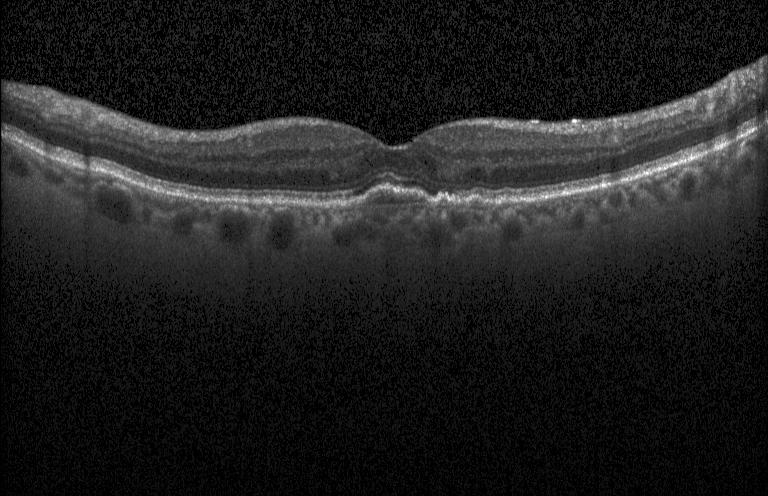 Retinal OCT cross-section; centered on the fovea; spectral-domain OCT.
Assessment: a choroidal neovascular membrane.